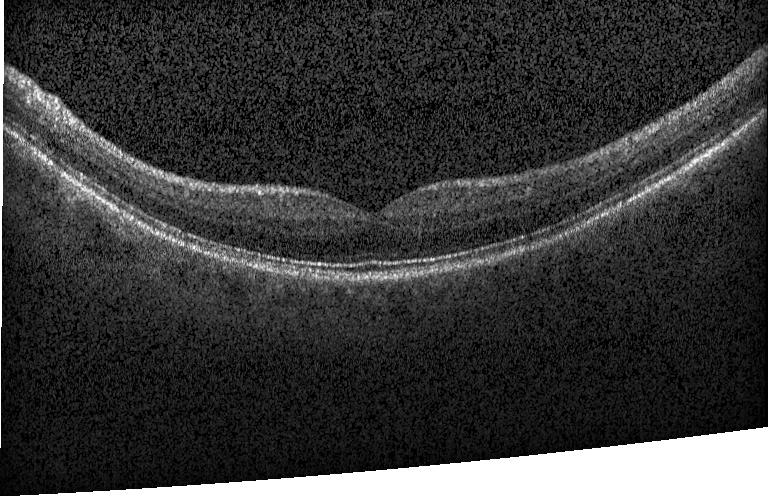 Spectral-domain OCT. Macular scan. Optical coherence tomography B-scan. Assessment: neither choroidal neovascularization, diabetic macular edema, nor drusen.